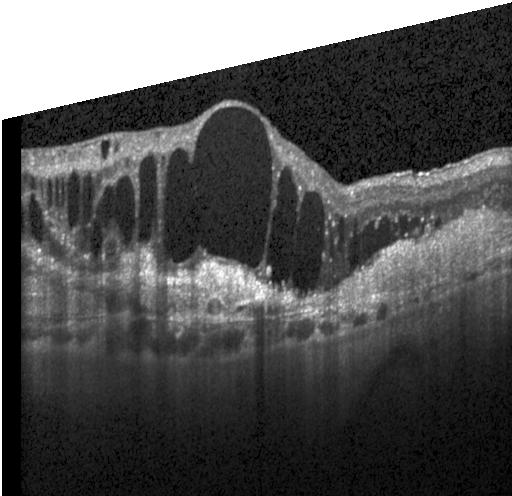

Instrument: Heidelberg Spectralis. Optical coherence tomography B-scan. Spectral-domain optical coherence tomography. Centered on the fovea
OCT finding: choroidal neovascularization.